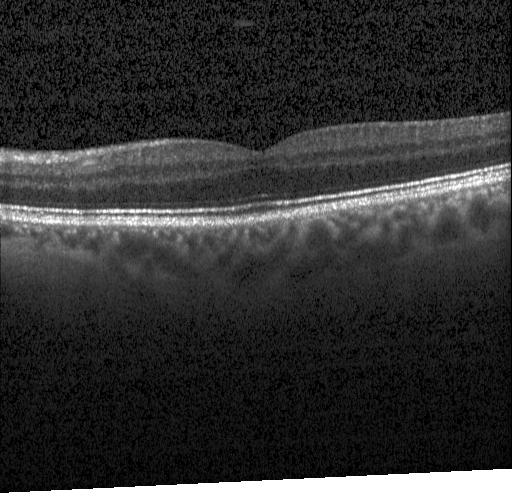
Optical coherence tomography scan. Finding: neither choroidal neovascularization, diabetic macular edema, nor drusen.